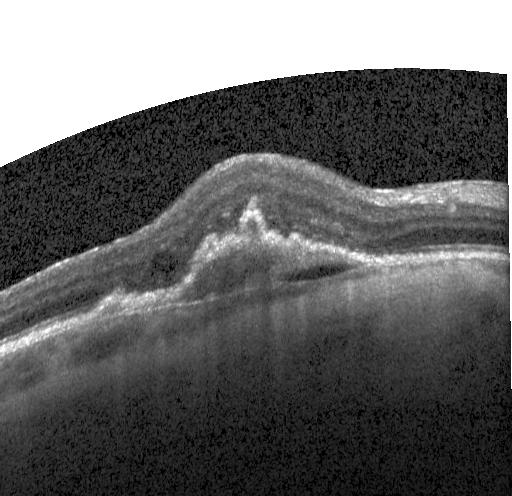
Assessment: a choroidal neovascular membrane.